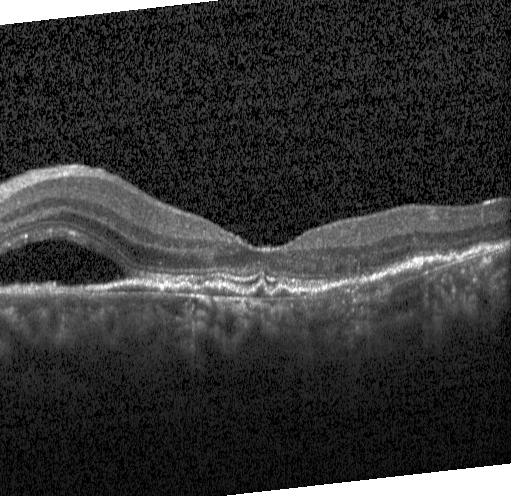 OCT line scan, macular scan
This B-scan demonstrates CNV.